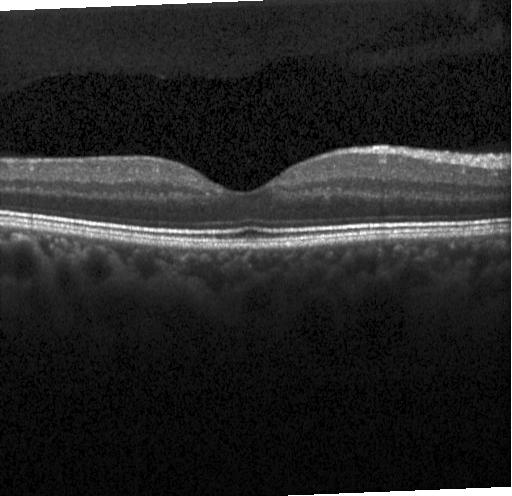

SD-OCT. Instrument: Heidelberg Spectralis. Macular scan. Optical coherence tomography B-scan.
Assessment: no choroidal neovascularization, diabetic macular edema, or drusen.